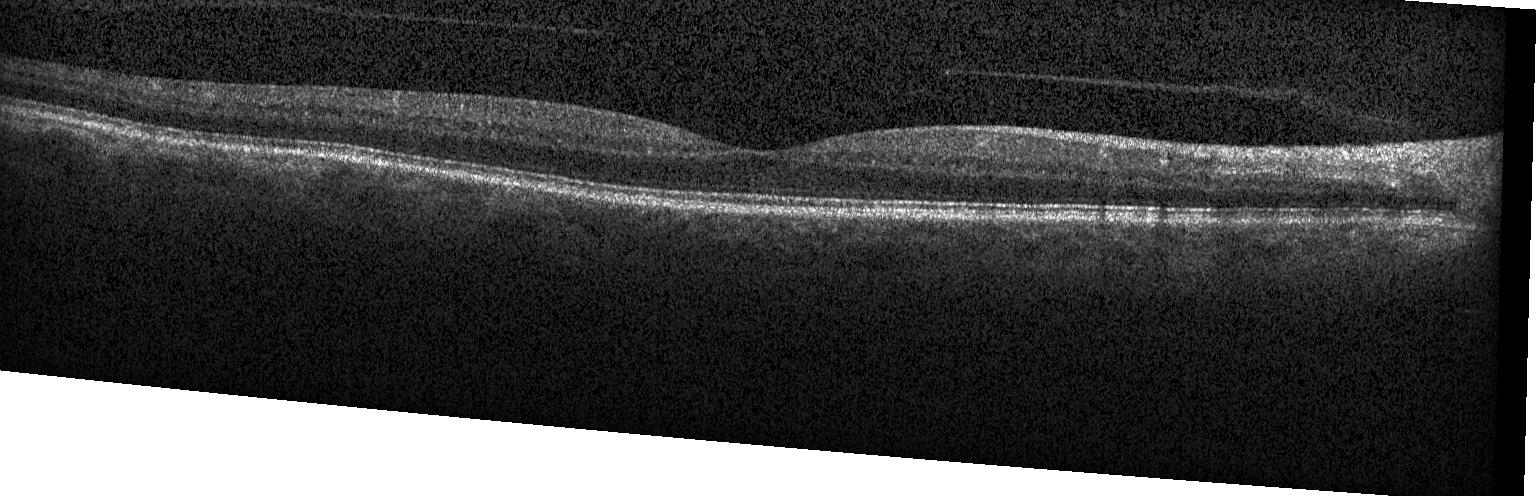 Spectral-domain OCT B-scan: no choroidal neovascularization, diabetic macular edema, or drusen.